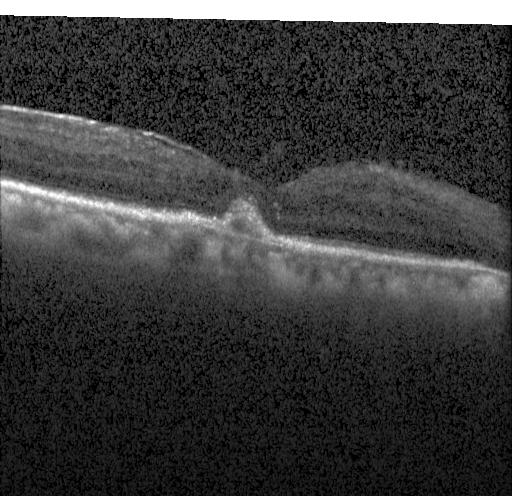

Macular OCT demonstrating choroidal neovascularization.